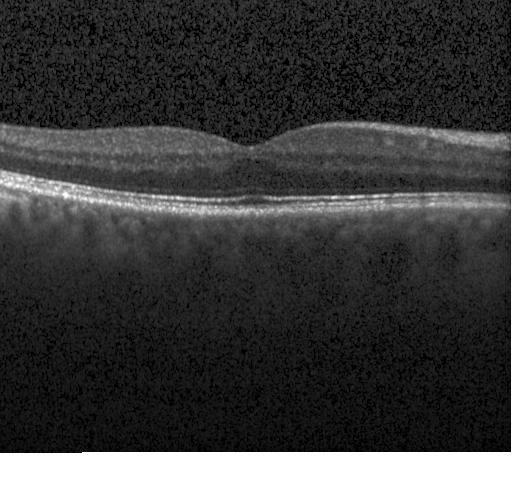
Horizontal scan through the fovea; optical coherence tomography scan. Impression: neither choroidal neovascularization, diabetic macular edema, nor drusen.